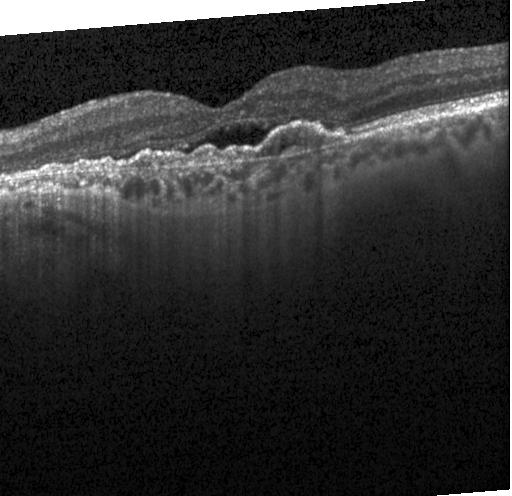

Assessment: choroidal neovascularization (CNV).